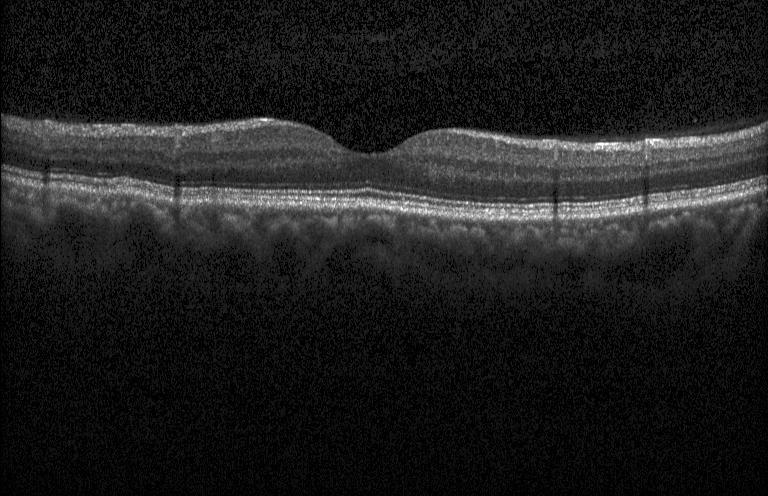
Retinal OCT cross-section showing no evidence of CNV, DME, or drusen.